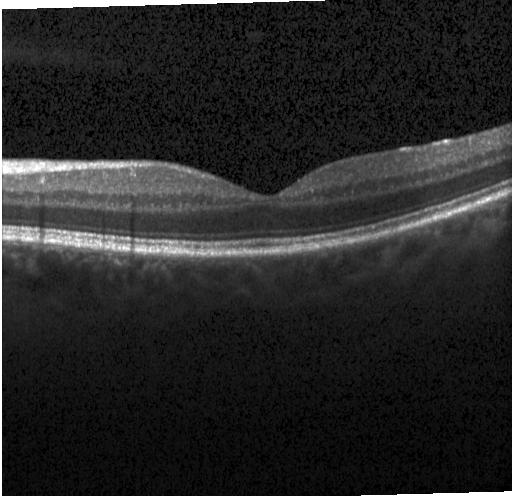 OCT B-scan. Spectral-domain optical coherence tomography
Assessment: neither choroidal neovascularization, diabetic macular edema, nor drusen.